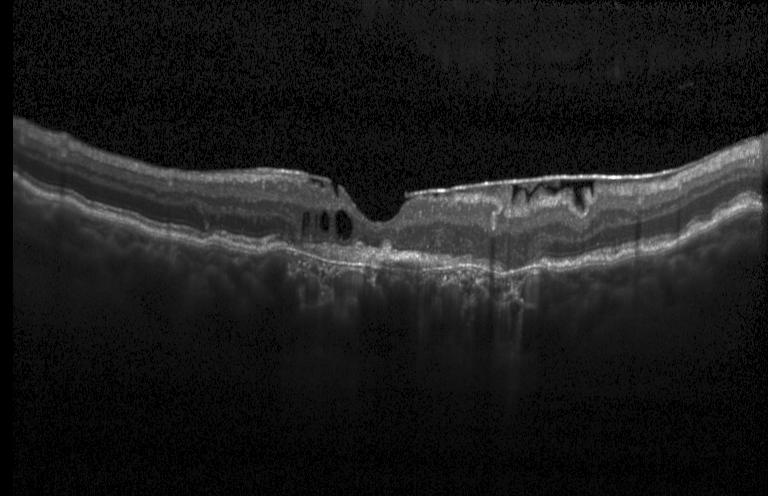
Retinal OCT cross-section · macular scan · spectral-domain OCT.
The scan shows a choroidal neovascular membrane.